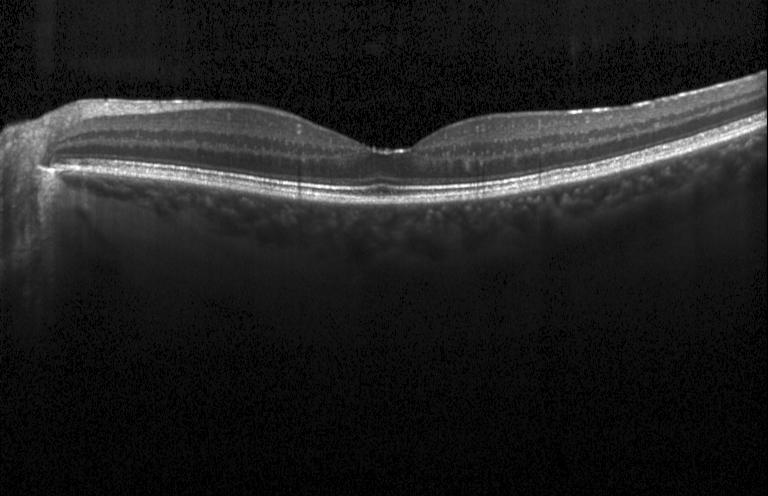
Retinal OCT cross-section showing no evidence of CNV, DME, or drusen.